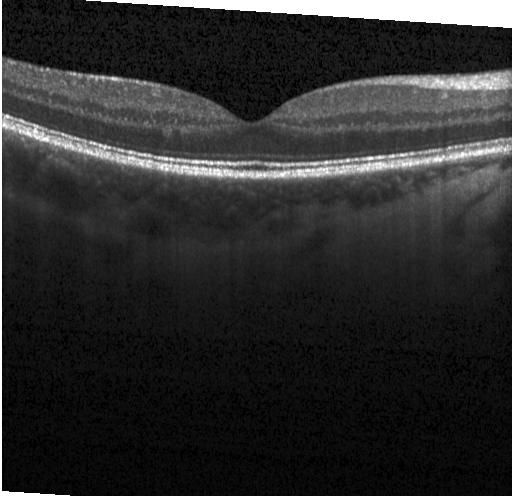

Macular scan · Heidelberg Spectralis OCT system · optical coherence tomography B-scan
Diagnosis: no CNV, DME, or drusen.